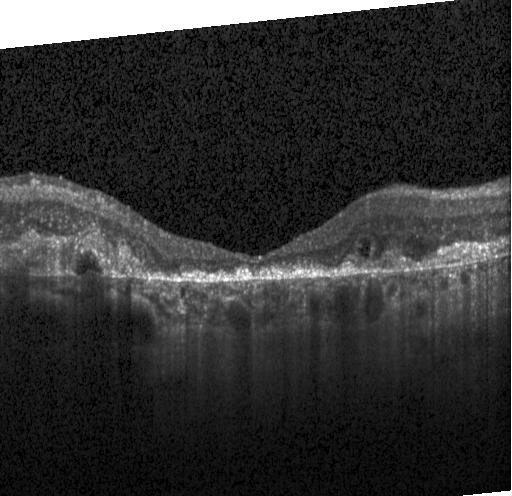 Assessment: choroidal neovascularization (CNV).